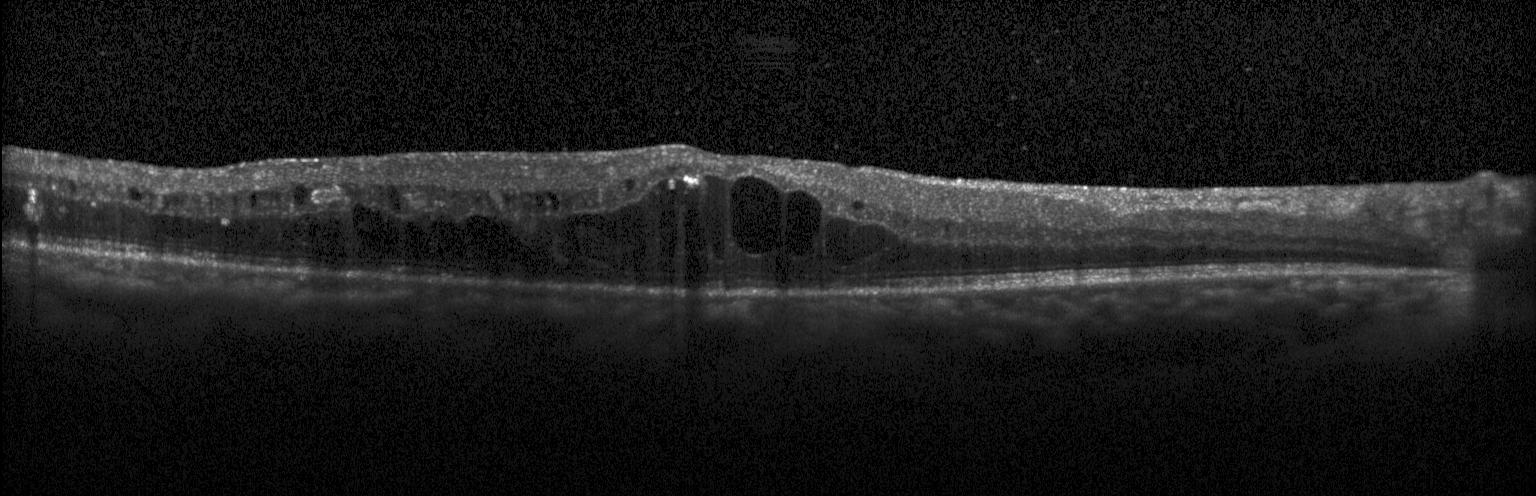

Diagnosis: diabetic macular edema (DME).